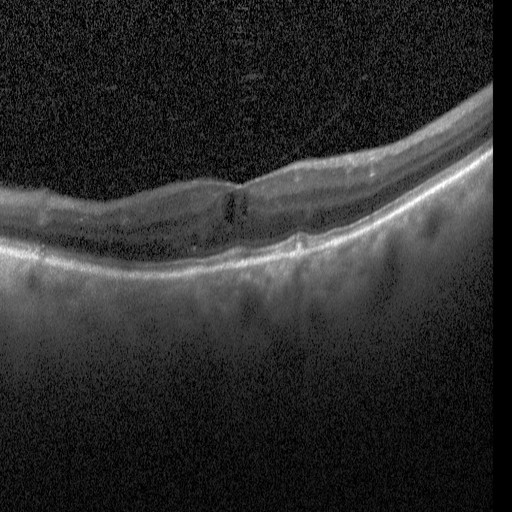
OCT finding: diabetic macular edema (DME).